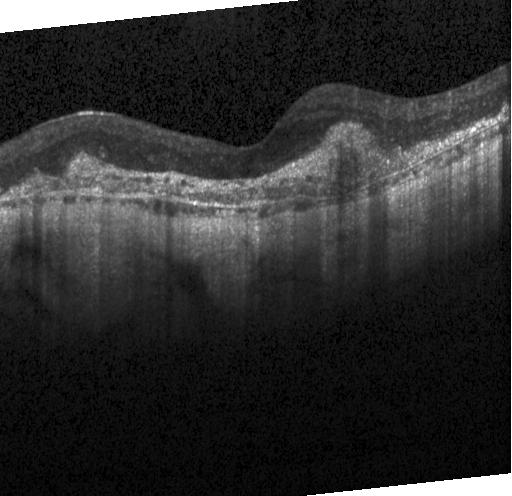

Macular OCT: CNV.